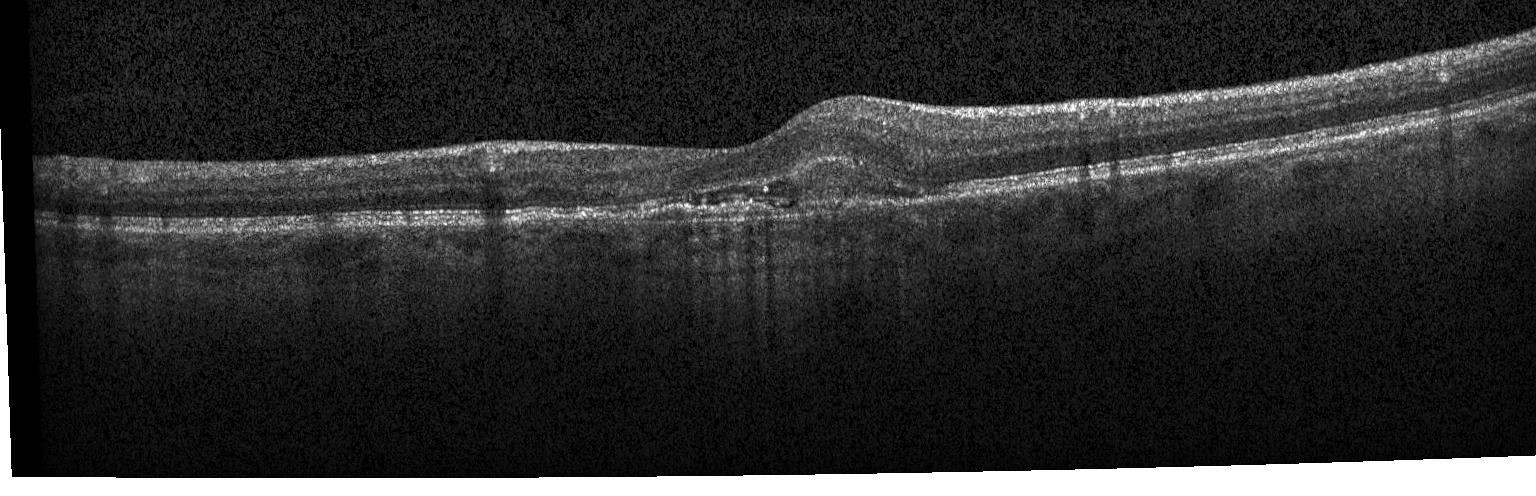 Spectral-domain OCT, centered on the fovea, retinal OCT cross-section
Impression: CNV.